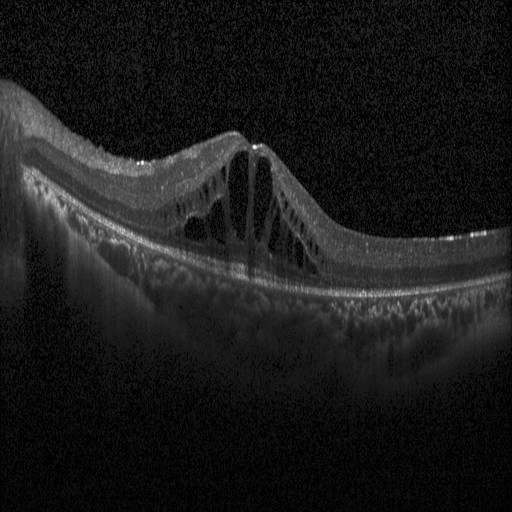

Retinal OCT cross-section; centered on the fovea; acquired on a Heidelberg Spectralis
Impression: DME.